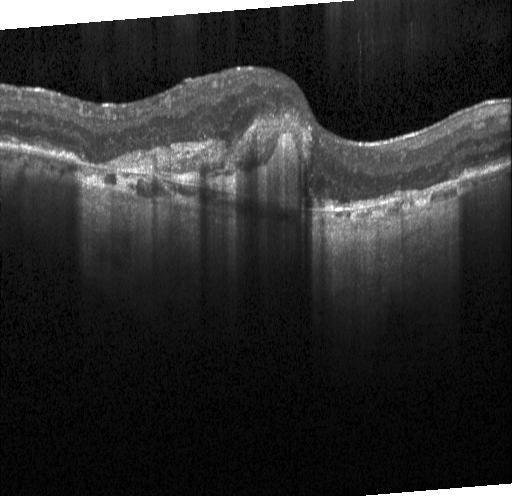 OCT finding: choroidal neovascularization (CNV).